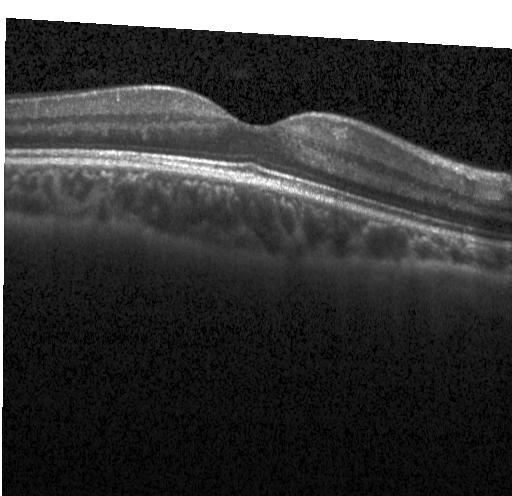 Centered on the fovea; OCT line scan
Finding: no choroidal neovascularization, no diabetic macular edema, and no drusen.